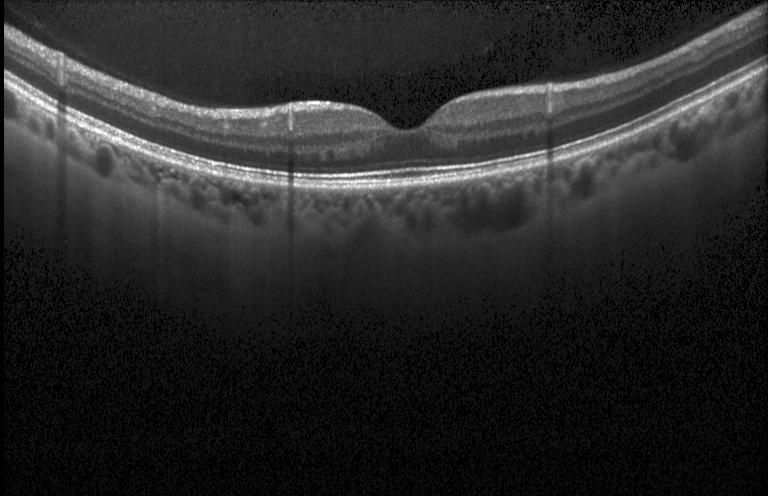 Finding: neither CNV, DME, nor drusen.